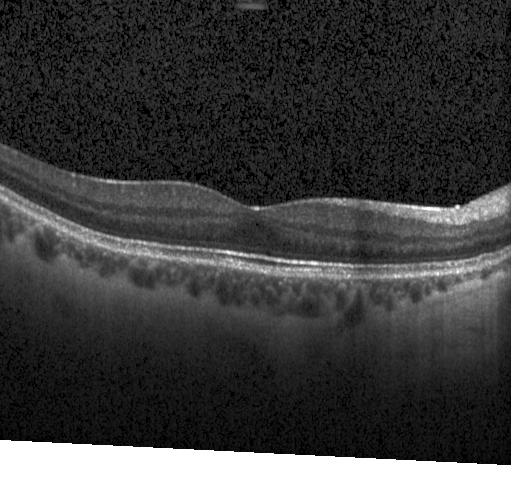

Macular OCT: no CNV, no DME, and no drusen.